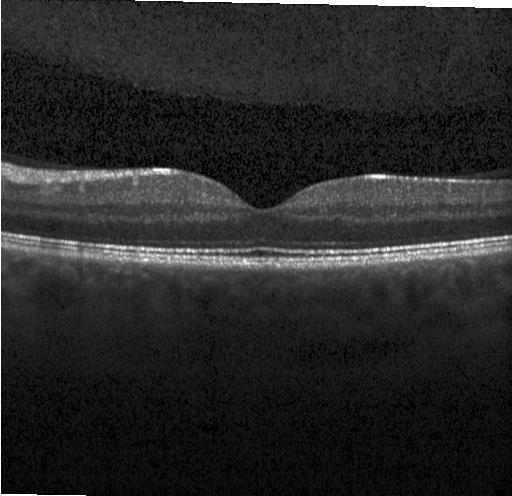
OCT B-scan.
Finding: no evidence of choroidal neovascularization, diabetic macular edema, or drusen.